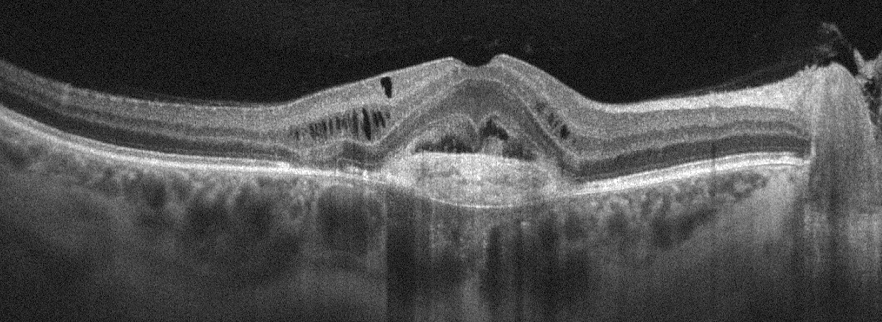

Right eye, retinal OCT B-scan.
Macular OCT: age-related macular degeneration (AMD).